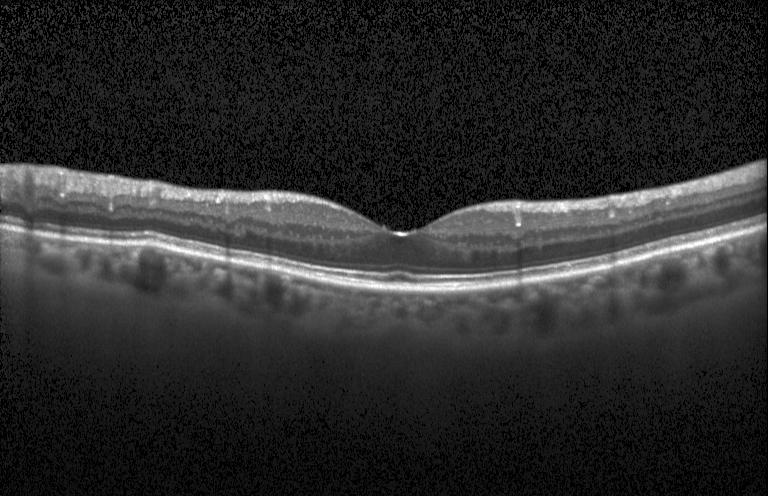
Optical coherence tomography scan. Macular OCT: no CNV, no DME, and no drusen.